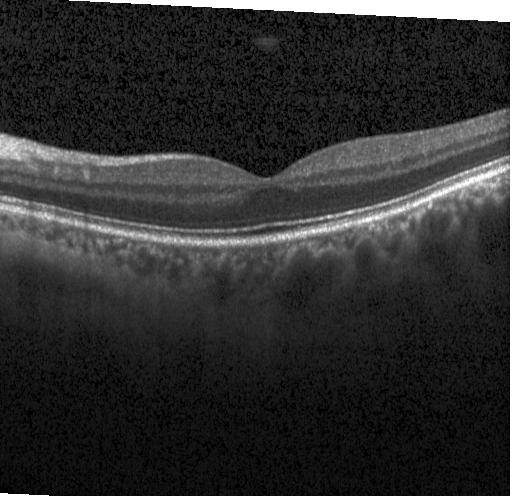
Horizontal scan through the fovea · instrument: Heidelberg Spectralis · OCT line scan
Finding: no evidence of choroidal neovascularization, diabetic macular edema, or drusen.